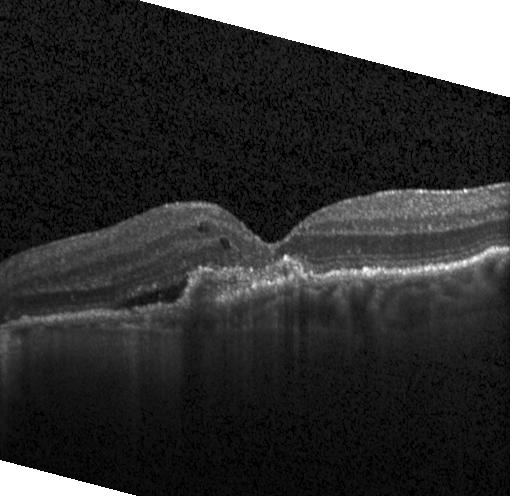

Assessment: a choroidal neovascular membrane.